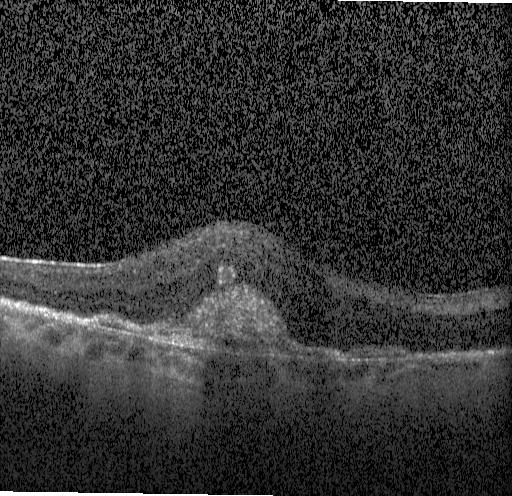 Instrument: Heidelberg Spectralis; macular scan; optical coherence tomography B-scan; spectral-domain optical coherence tomography.
Finding: CNV.